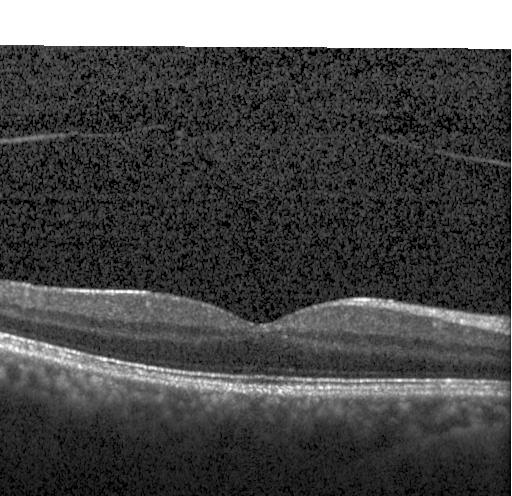

Retinal OCT cross-section · spectral-domain optical coherence tomography. OCT finding: no CNV, DME, or drusen.